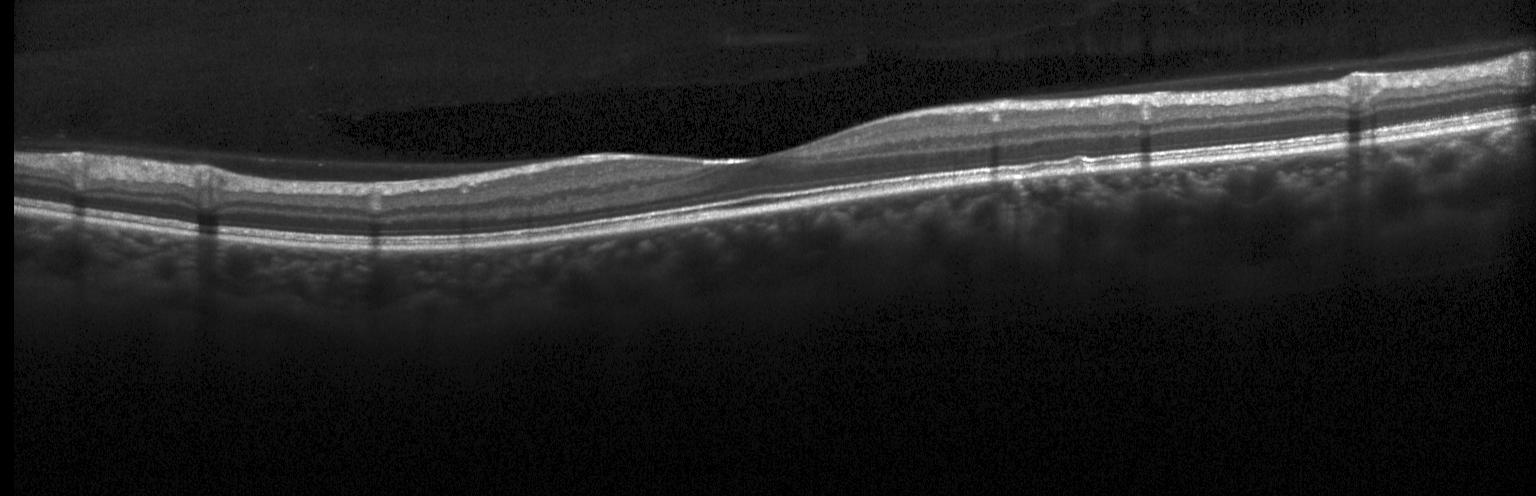 Finding: no CNV, DME, or drusen.